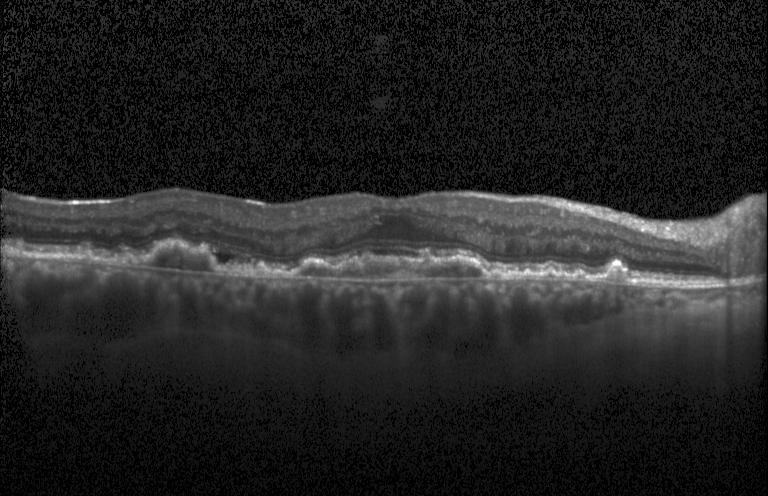
This B-scan demonstrates choroidal neovascularization.